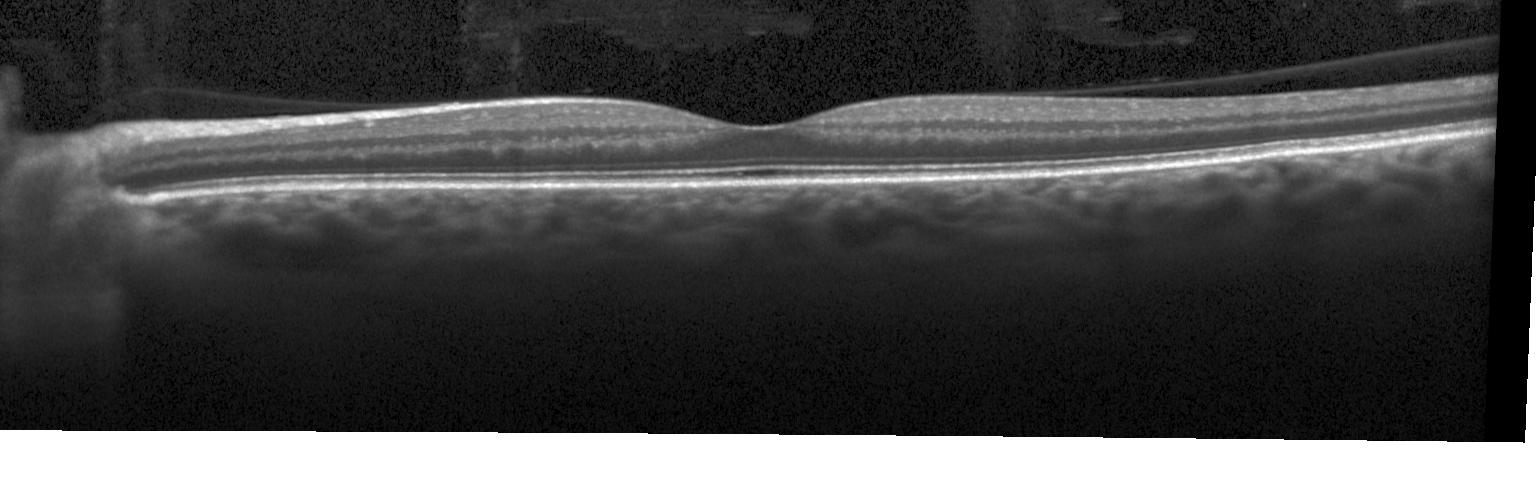 OCT B-scan showing no CNV, no DME, and no drusen.